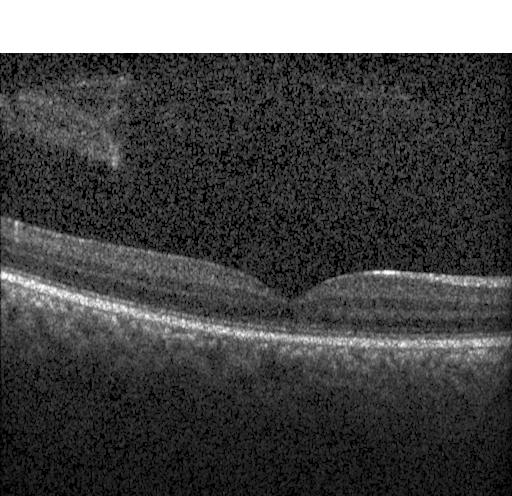 OCT line scan, spectral-domain optical coherence tomography.
Impression: neither CNV, DME, nor drusen.